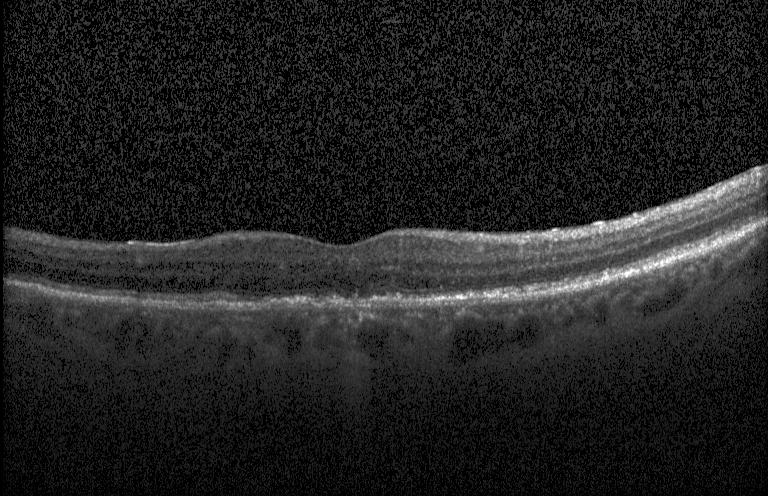
Centered on the fovea; optical coherence tomography scan; instrument: Heidelberg Spectralis.
Impression: CNV.